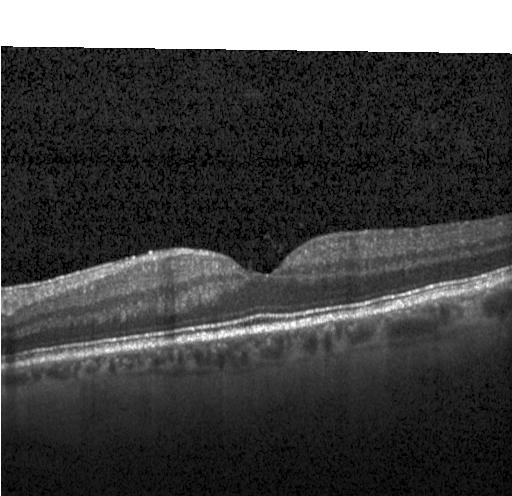

Macular scan, optical coherence tomography scan, Heidelberg Spectralis OCT system, spectral-domain OCT.
Neither choroidal neovascularization, diabetic macular edema, nor drusen.